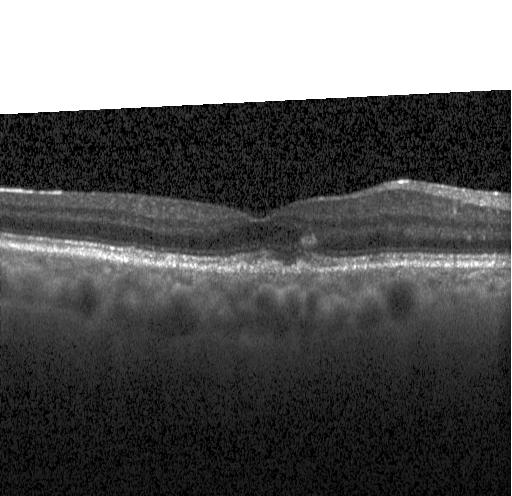
OCT line scan — Diagnosis: multiple drusen.